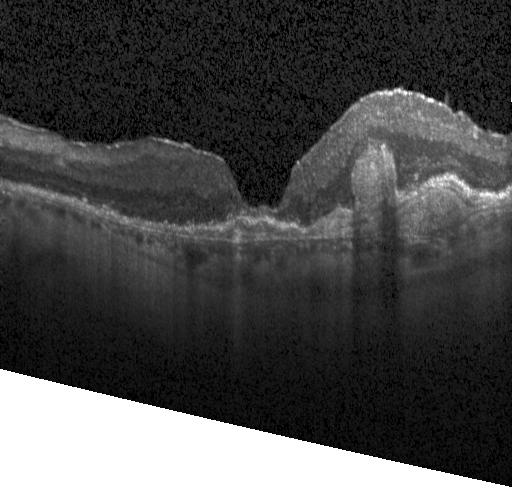

Macular scan, Heidelberg Spectralis, SD-OCT, OCT line scan
This B-scan demonstrates choroidal neovascularization (CNV).